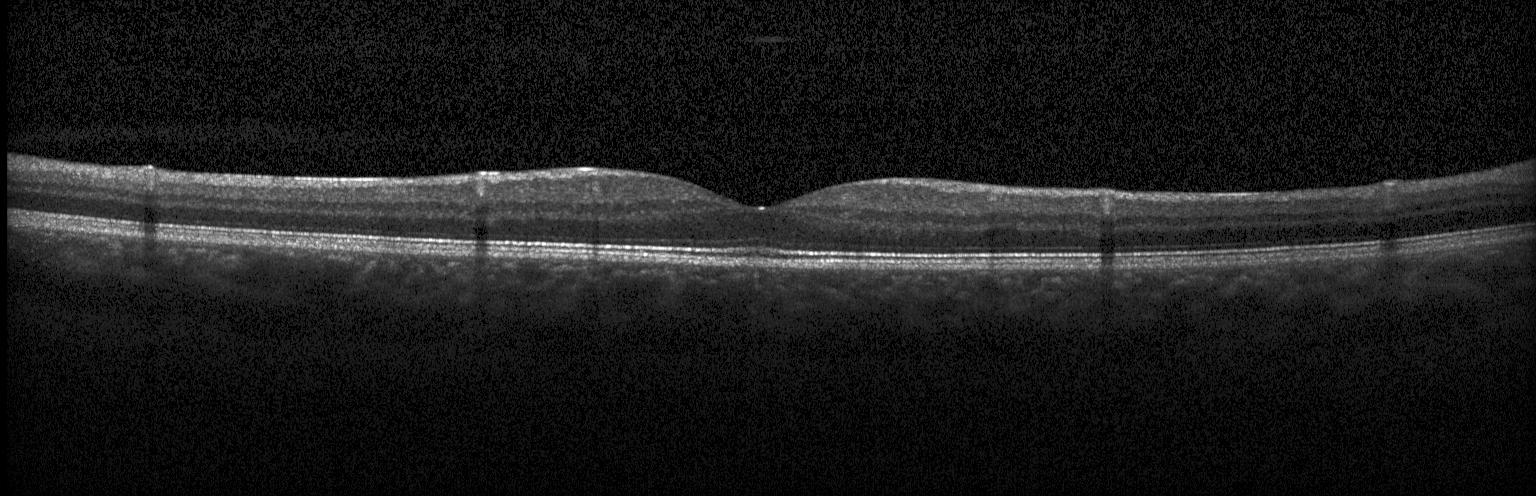
Dx: neither CNV, DME, nor drusen.